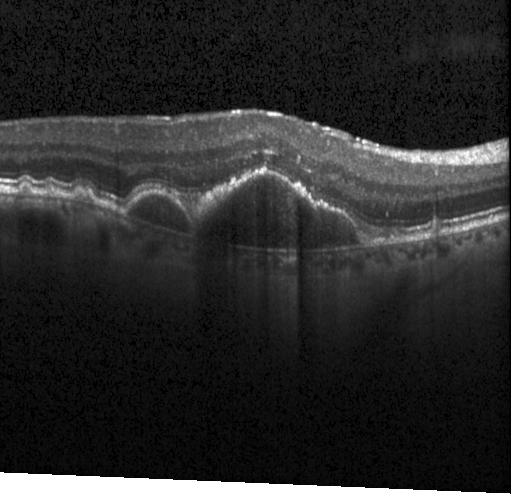
Fovea-centered; SD-OCT; Heidelberg Spectralis OCT system; OCT B-scan. Diagnosis: a choroidal neovascular membrane.